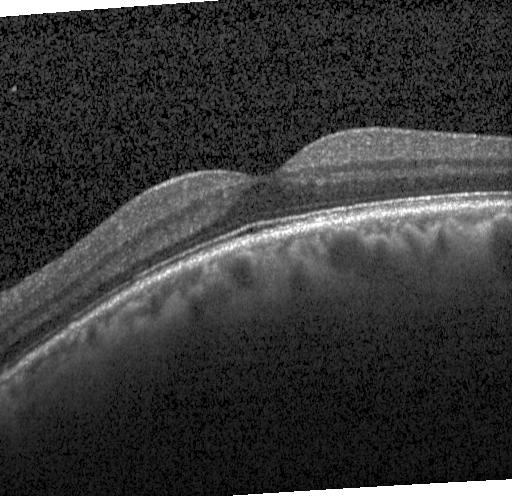
OCT scan showing neither CNV, DME, nor drusen.